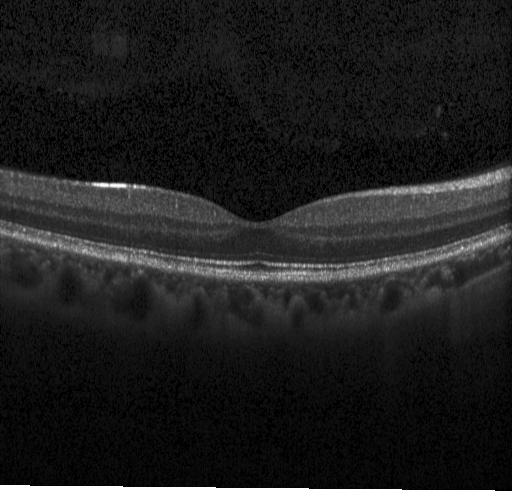
OCT line scan. Through the macula. Instrument: Heidelberg Spectralis. Spectral-domain OCT.
Dx: no choroidal neovascularization, no diabetic macular edema, and no drusen.